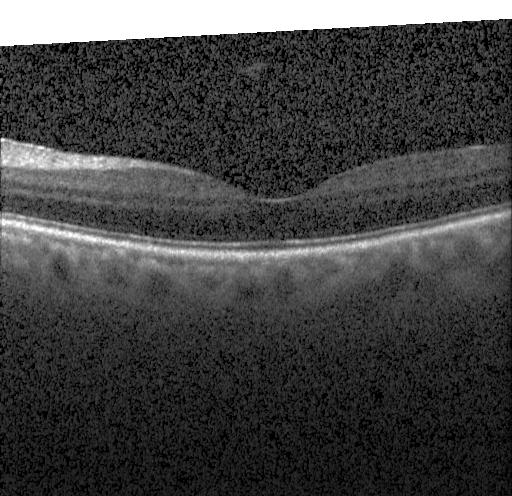 Heidelberg Spectralis OCT system, optical coherence tomography scan, macular scan, spectral-domain OCT.
Finding: no CNV, DME, or drusen.